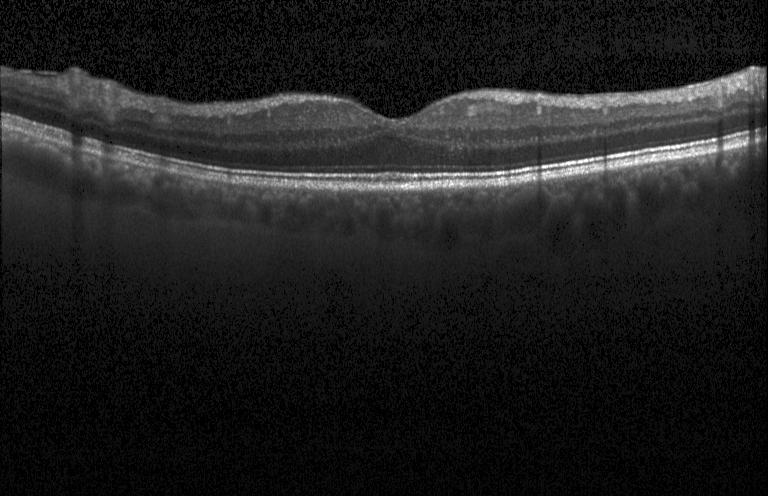 Heidelberg Spectralis; SD-OCT; centered on the fovea; optical coherence tomography B-scan.
Diagnosis: neither CNV, DME, nor drusen.